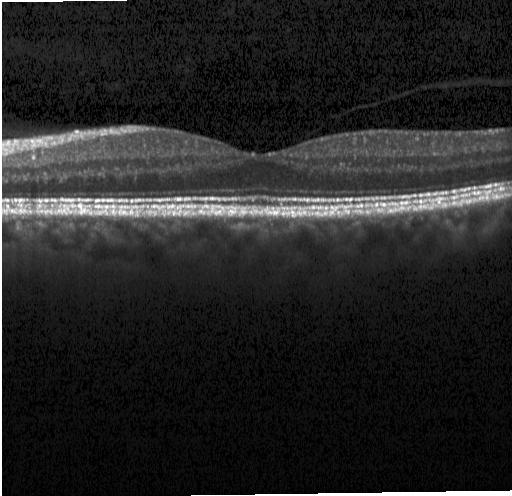

OCT line scan.
Dx: neither CNV, DME, nor drusen.